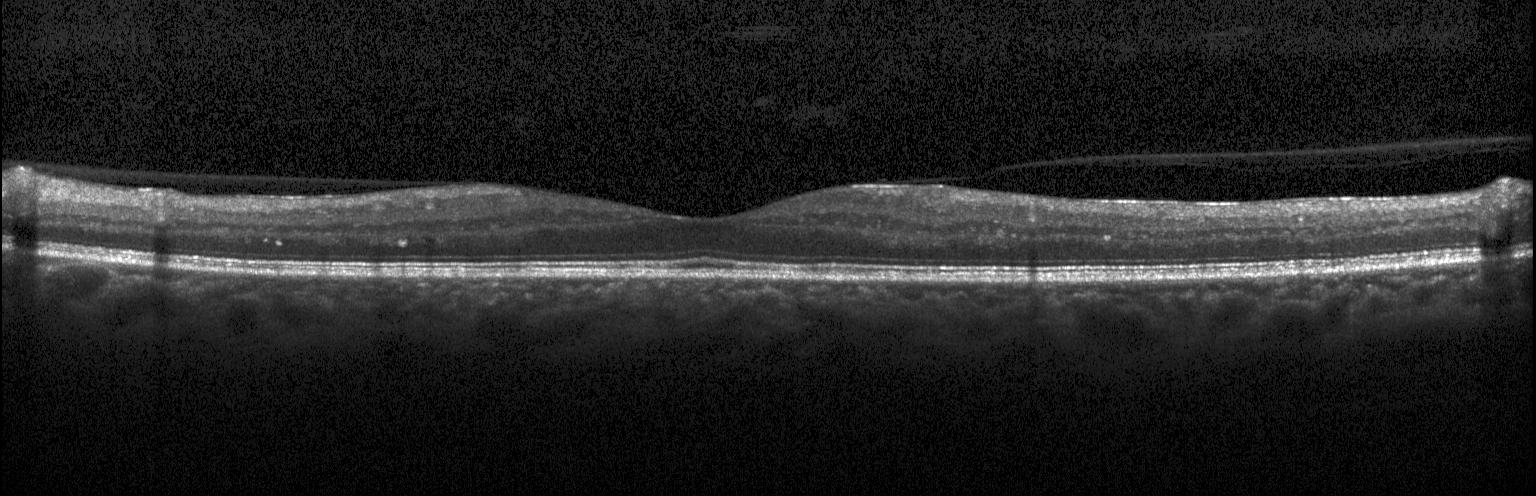

Acquired on a Heidelberg Spectralis, macular scan, spectral-domain OCT, OCT line scan
Neither choroidal neovascularization, diabetic macular edema, nor drusen.